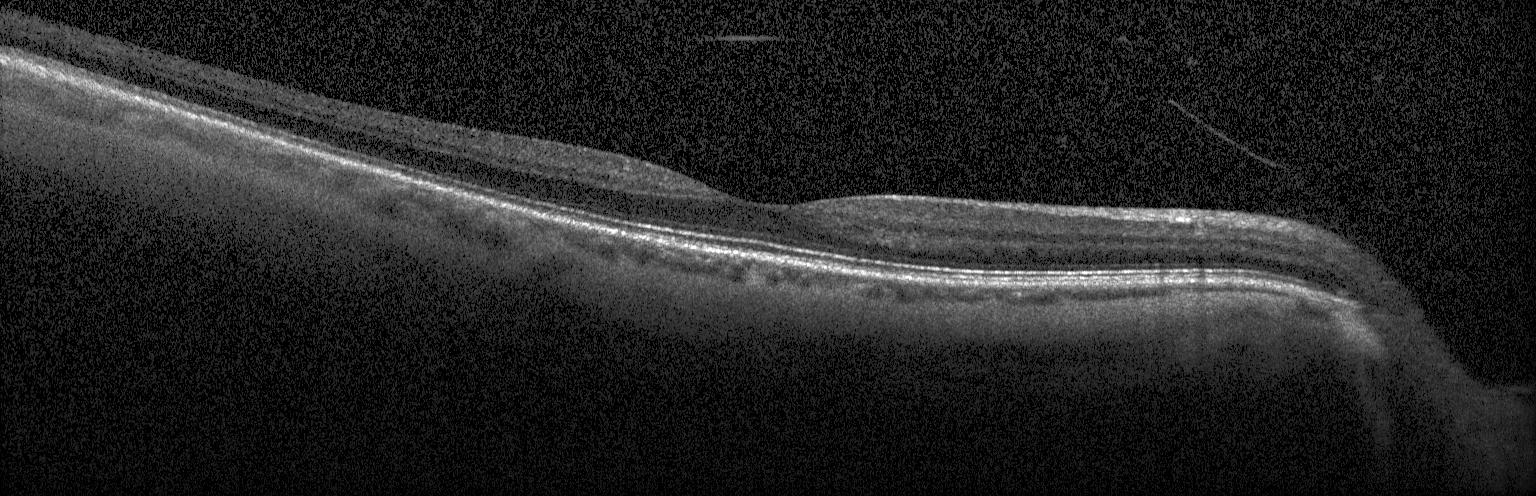

Impression: no choroidal neovascularization, diabetic macular edema, or drusen.